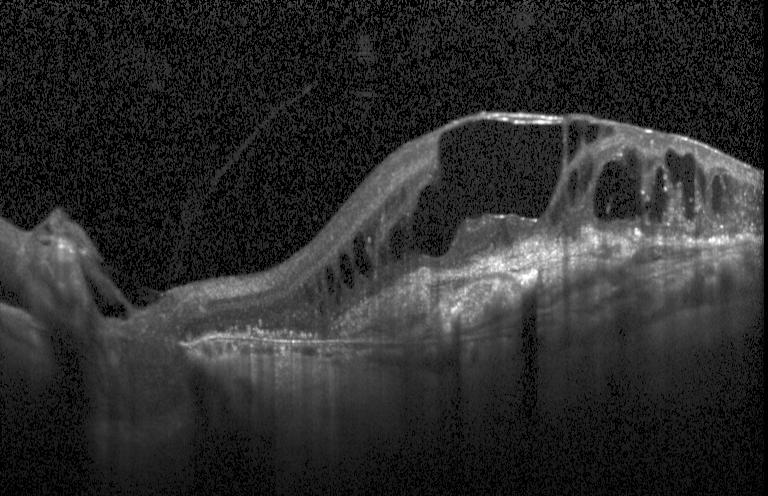 Retinal OCT B-scan.
Dx: a choroidal neovascular membrane.